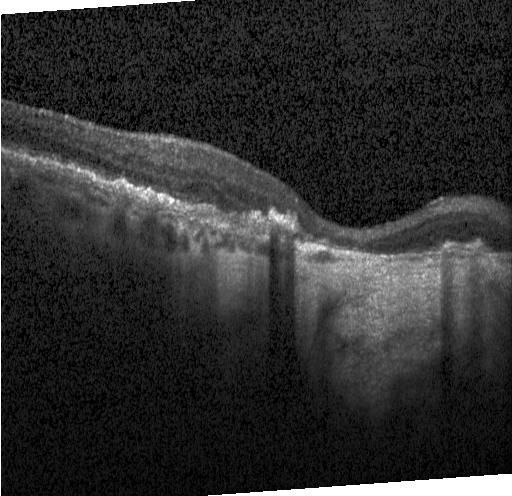
OCT scan showing a choroidal neovascular membrane.